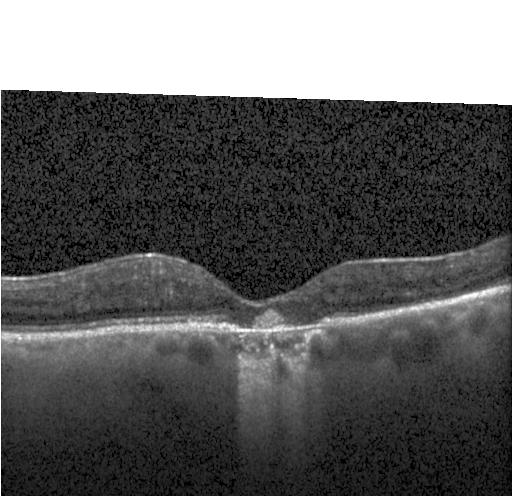

OCT finding: CNV.